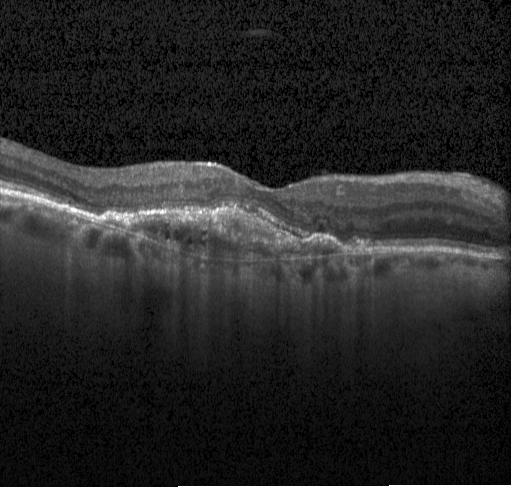

OCT B-scan
Dx: choroidal neovascularization.